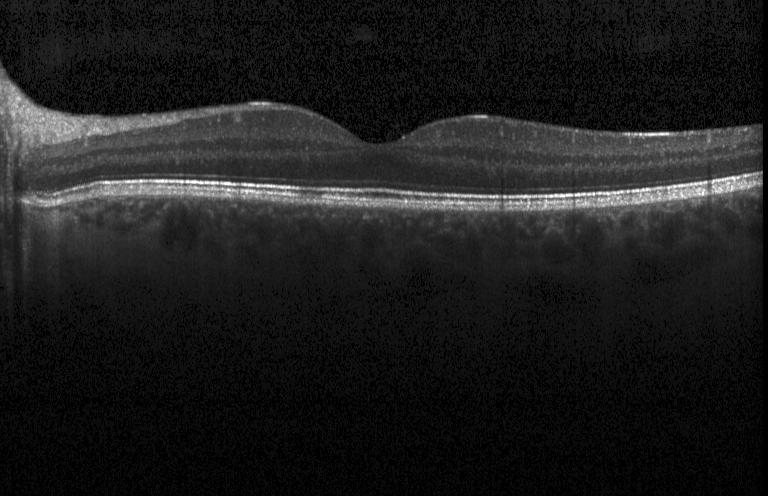 Spectral-domain OCT · fovea-centered · OCT B-scan · Heidelberg Spectralis. Diagnosis: no evidence of choroidal neovascularization, diabetic macular edema, or drusen.